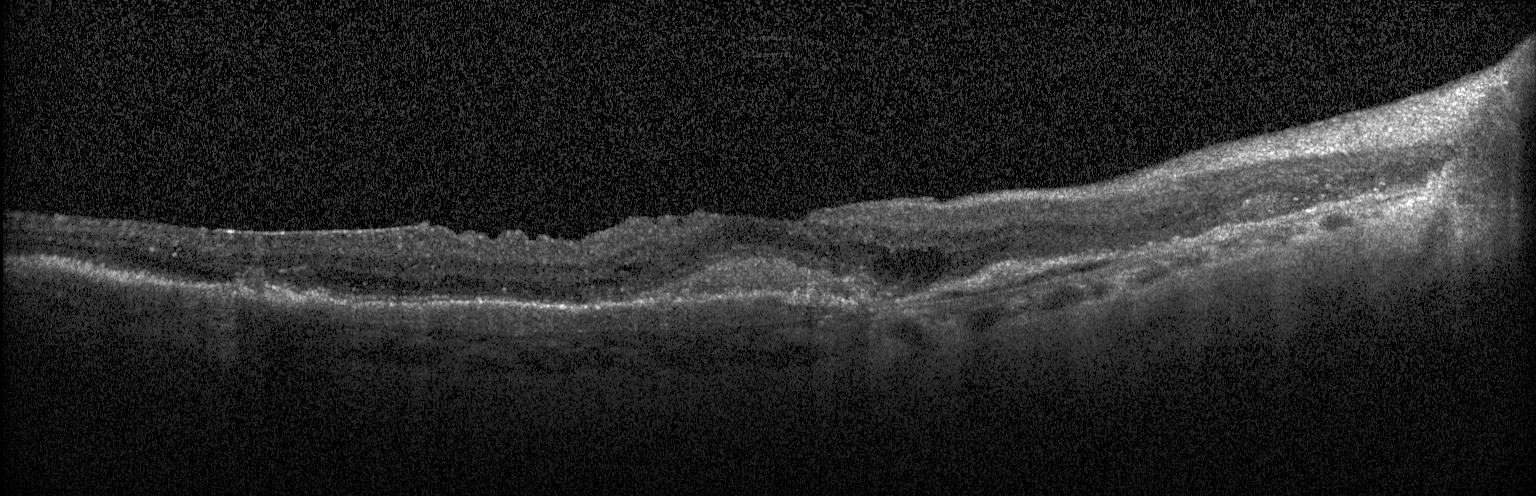

Centered on the fovea, OCT B-scan, spectral-domain OCT.
The scan shows CNV.